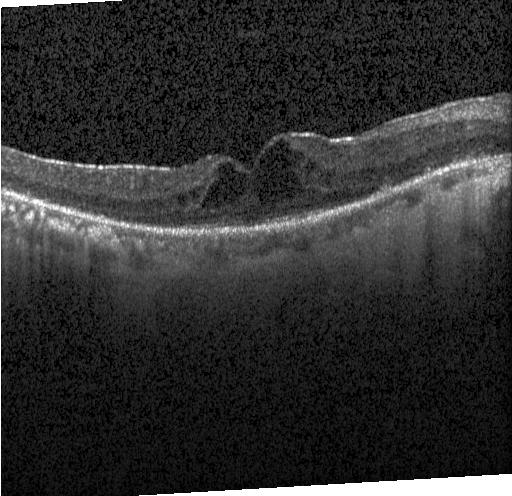 Finding: DME.